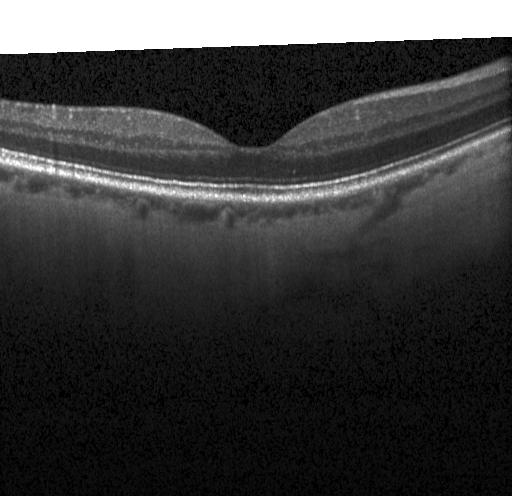

Spectral-domain OCT · centered on the fovea · retinal OCT B-scan
Diagnosis: no evidence of CNV, DME, or drusen.